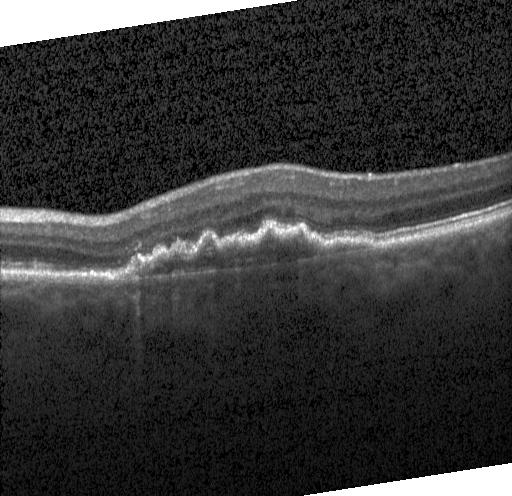
Instrument: Heidelberg Spectralis. OCT line scan.
Impression: a choroidal neovascular membrane.